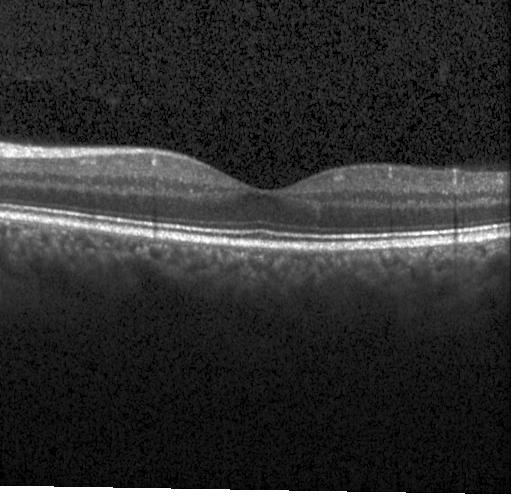
Retinal OCT cross-section showing neither choroidal neovascularization, diabetic macular edema, nor drusen.